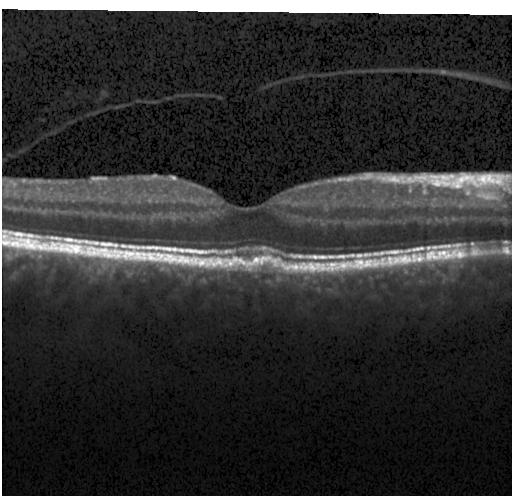 Dx: sub-RPE drusenoid deposits.